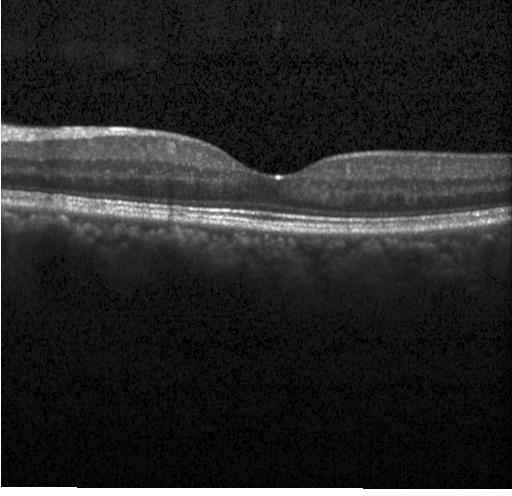 Instrument: Heidelberg Spectralis, centered on the fovea, retinal OCT cross-section — Finding: neither choroidal neovascularization, diabetic macular edema, nor drusen.